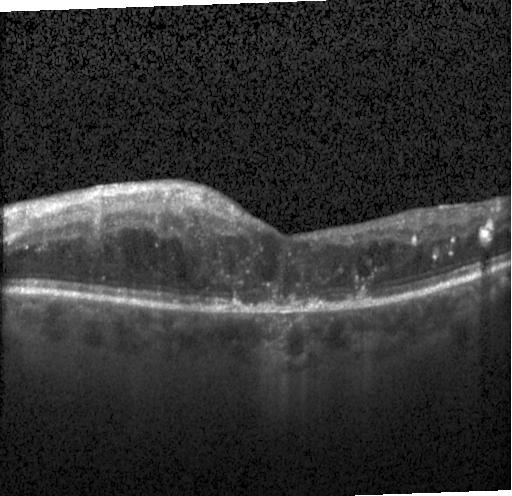
OCT B-scan
Diabetic macular edema (DME).